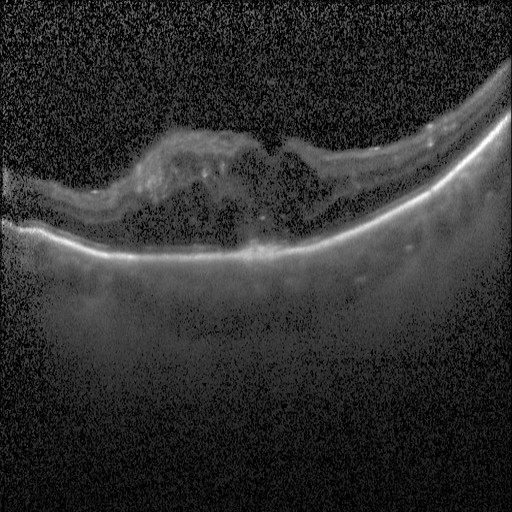 Horizontal scan through the fovea. OCT B-scan. Spectral-domain OCT. Acquired on a Heidelberg Spectralis — Macular OCT: DME.